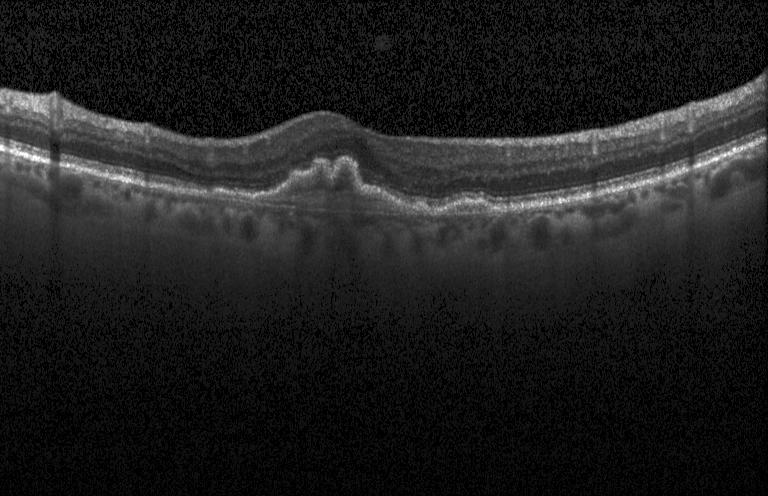
OCT scan showing CNV.